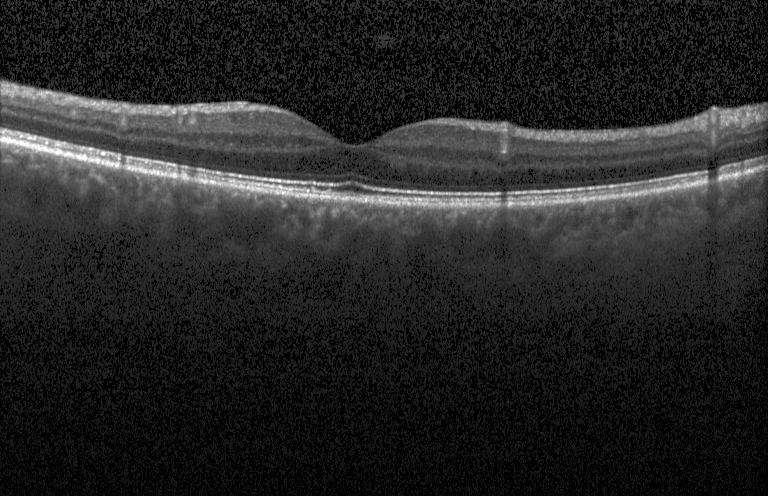 Finding: neither choroidal neovascularization, diabetic macular edema, nor drusen.